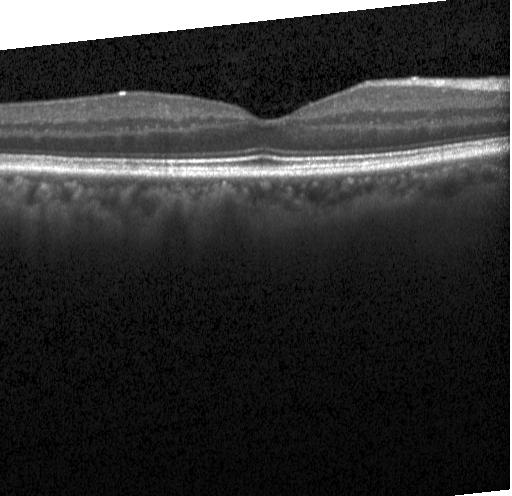 Spectral-domain optical coherence tomography · macular scan · OCT B-scan — Assessment: neither choroidal neovascularization, diabetic macular edema, nor drusen.